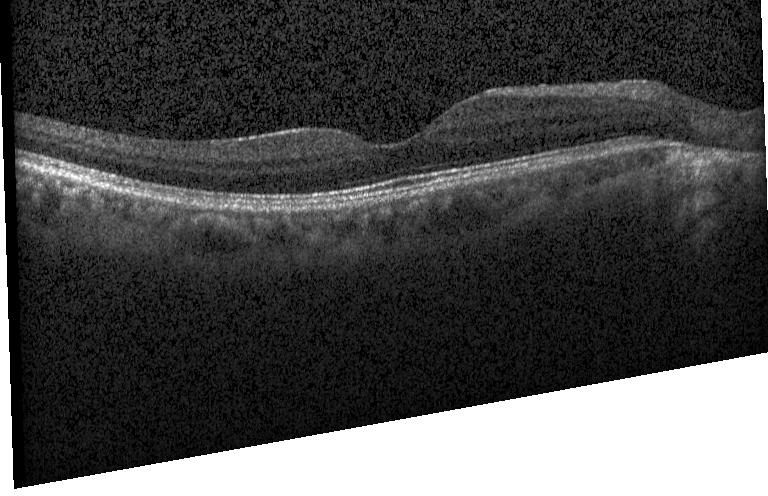
Centered on the fovea. Retinal OCT cross-section — Diagnosis: no evidence of choroidal neovascularization, diabetic macular edema, or drusen.